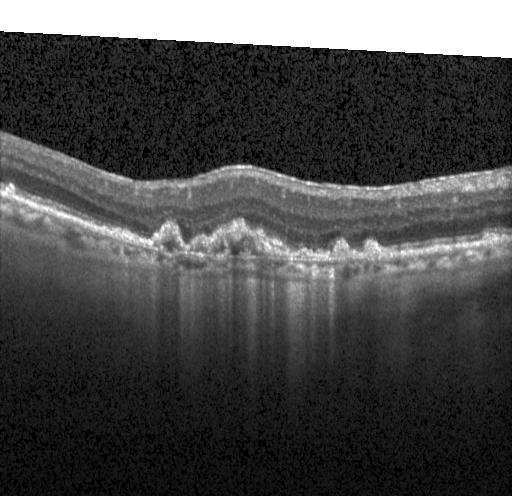 Macular OCT: a choroidal neovascular membrane.